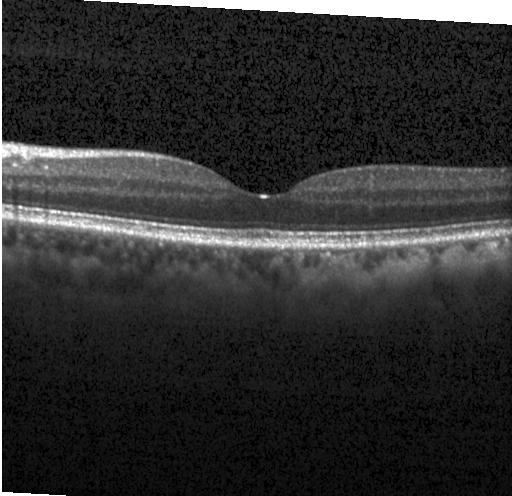

This B-scan demonstrates no evidence of CNV, DME, or drusen.